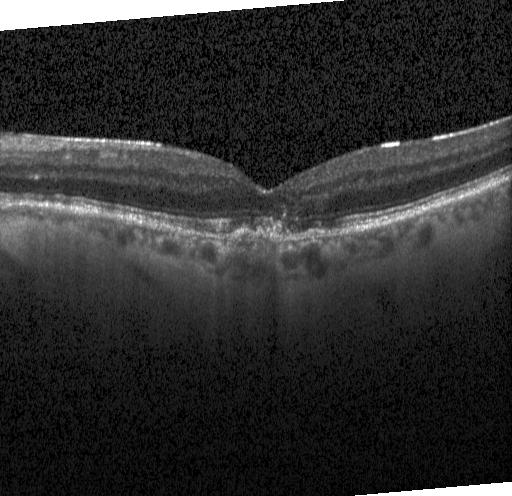 Choroidal neovascularization (CNV).